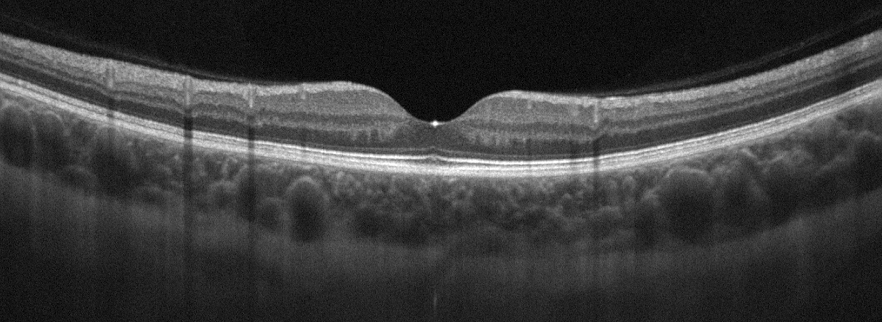
OCT B-scan · left eye. The scan shows absence of AMD, DME, ERM, RAO, RVO, and vitreomacular interface disease.